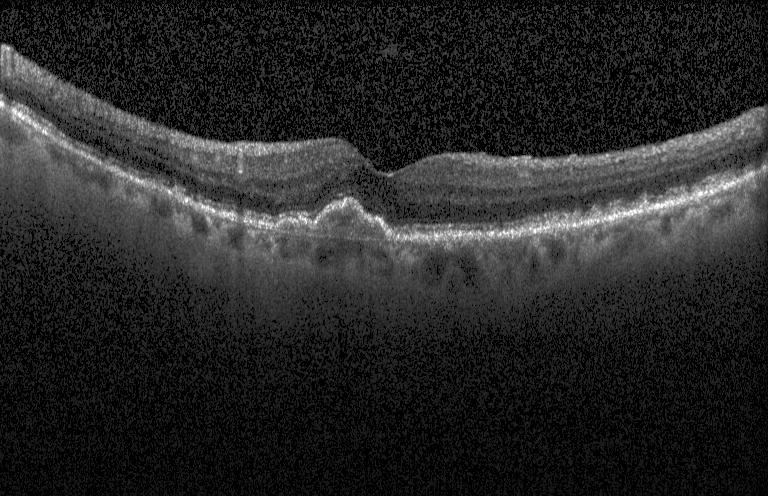
Retinal OCT B-scan — Impression: choroidal neovascularization.